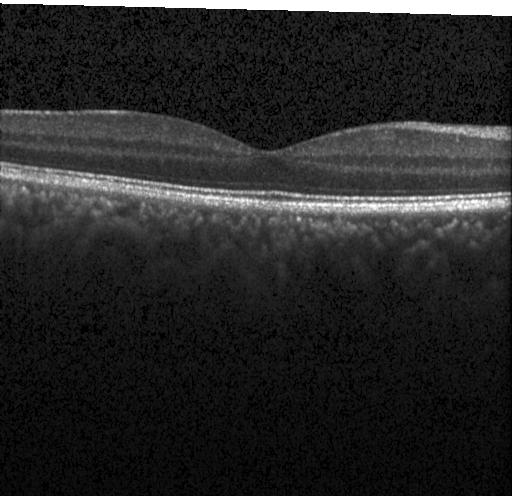

Macular scan; acquired on a Heidelberg Spectralis; OCT B-scan; spectral-domain optical coherence tomography.
Diagnosis: no CNV, DME, or drusen.